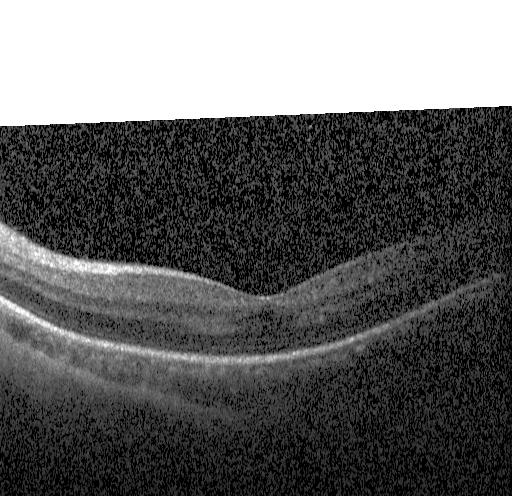 OCT line scan — Diagnosis: no evidence of CNV, DME, or drusen.